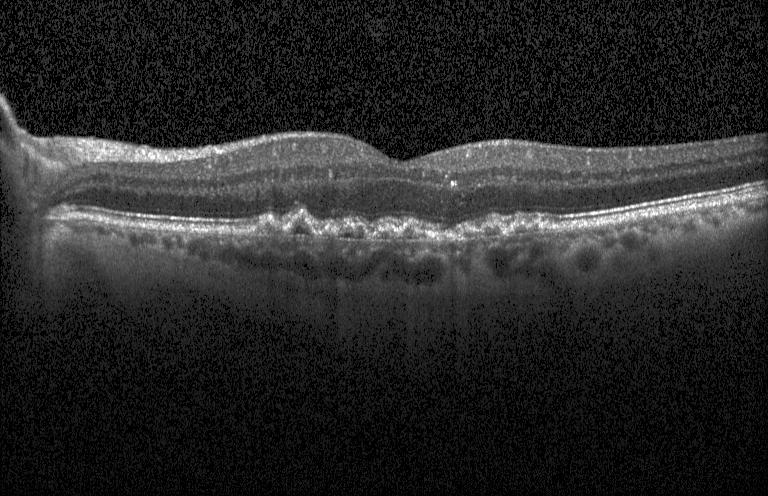
Assessment: sub-RPE drusenoid deposits.